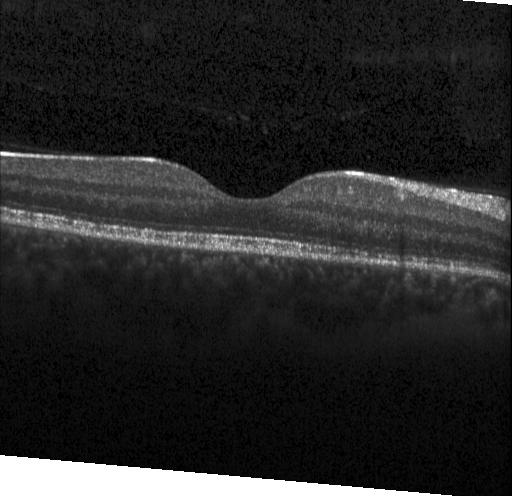

OCT finding: no CNV, no DME, and no drusen.